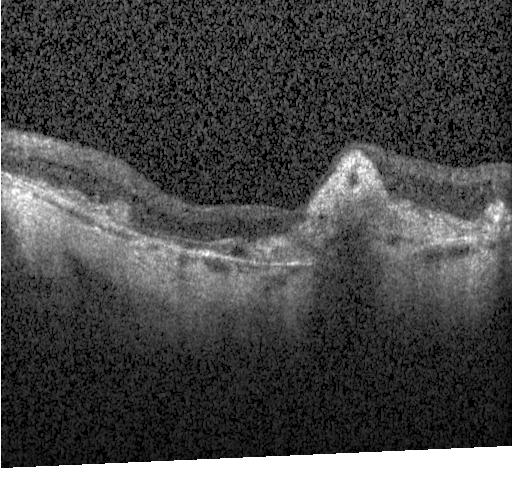 Optical coherence tomography scan; SD-OCT; macular scan.
This B-scan demonstrates a choroidal neovascular membrane.